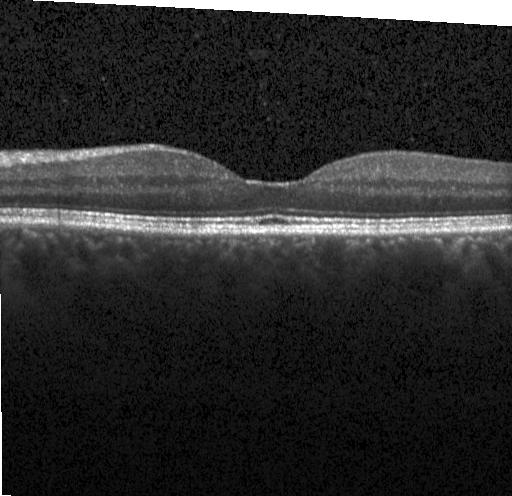

Heidelberg Spectralis. OCT B-scan. Finding: neither CNV, DME, nor drusen.